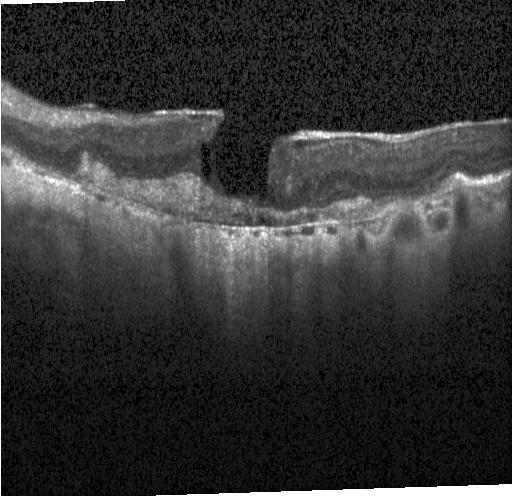 Retinal OCT cross-section — Impression: choroidal neovascularization (CNV).